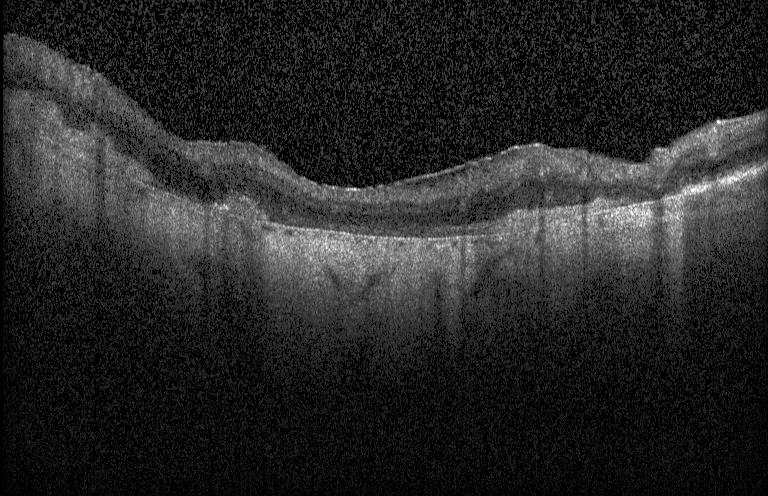

OCT finding: a choroidal neovascular membrane.